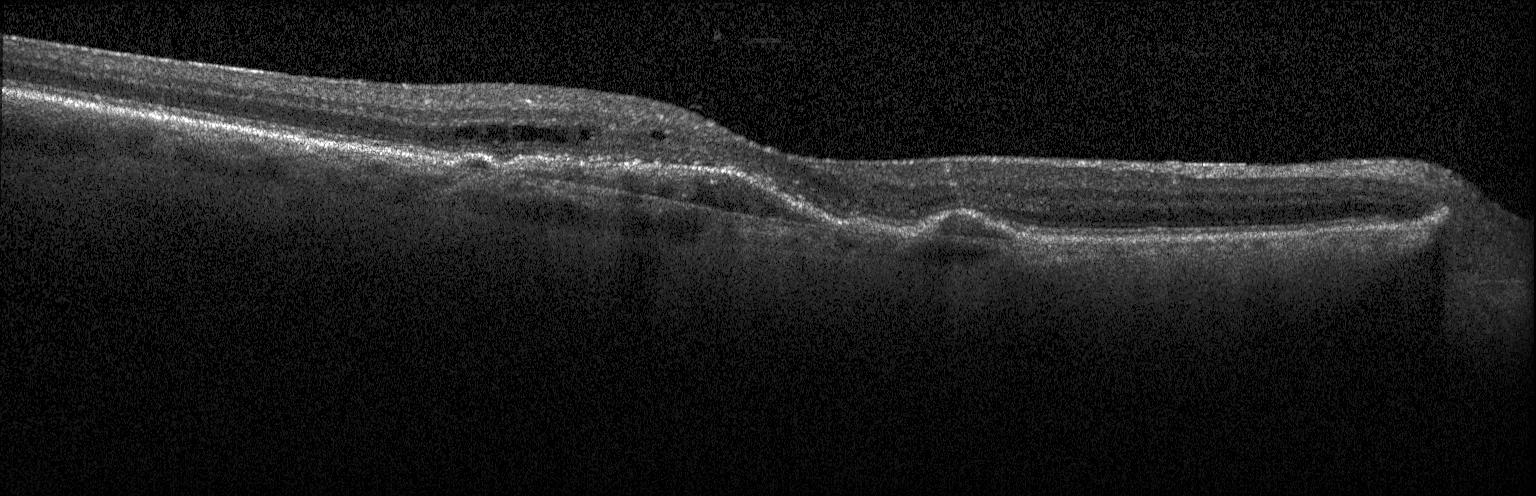

OCT B-scan.
Dx: CNV.